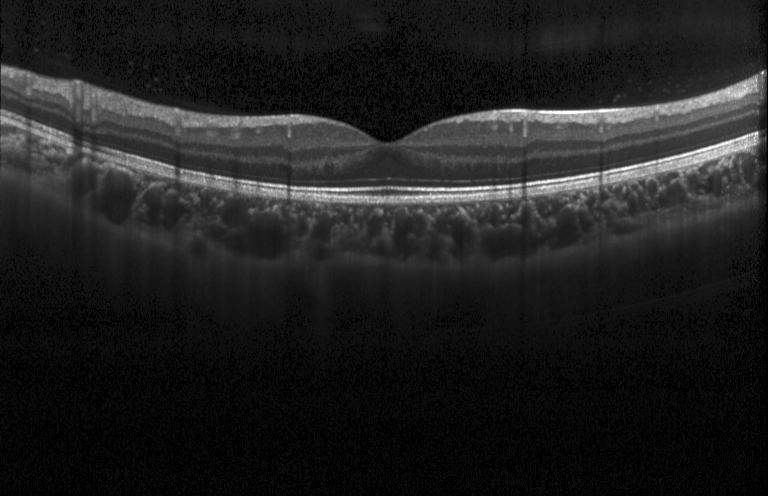

OCT B-scan. Through the macula — This B-scan demonstrates no evidence of CNV, DME, or drusen.